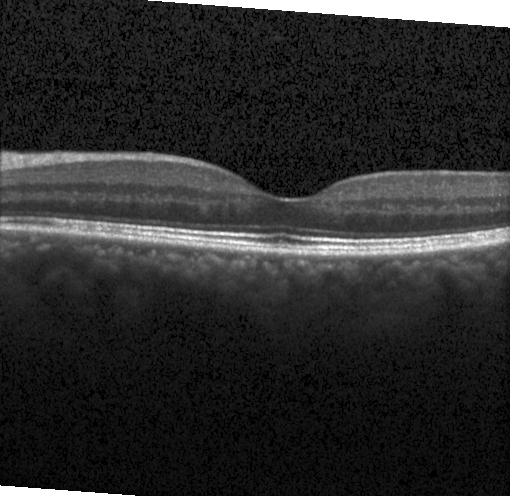
Spectral-domain OCT · fovea-centered · instrument: Heidelberg Spectralis · OCT B-scan.
OCT finding: no evidence of choroidal neovascularization, diabetic macular edema, or drusen.